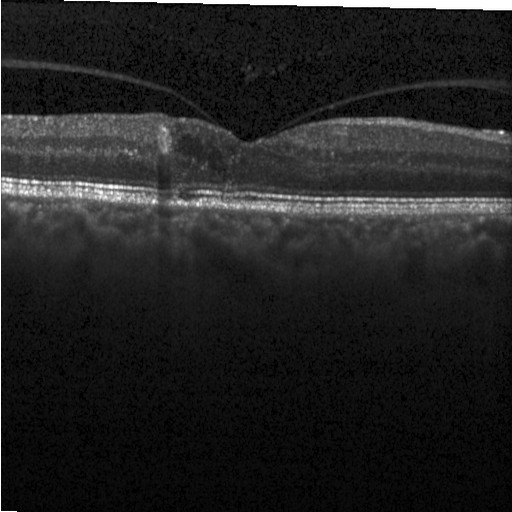

Horizontal scan through the fovea; OCT B-scan
Impression: DME.